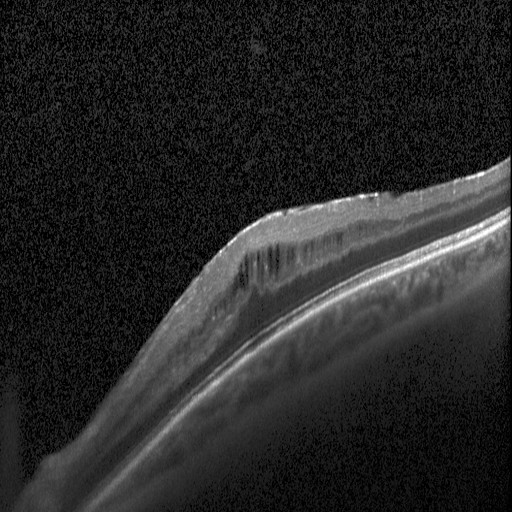

OCT finding: diabetic macular edema.